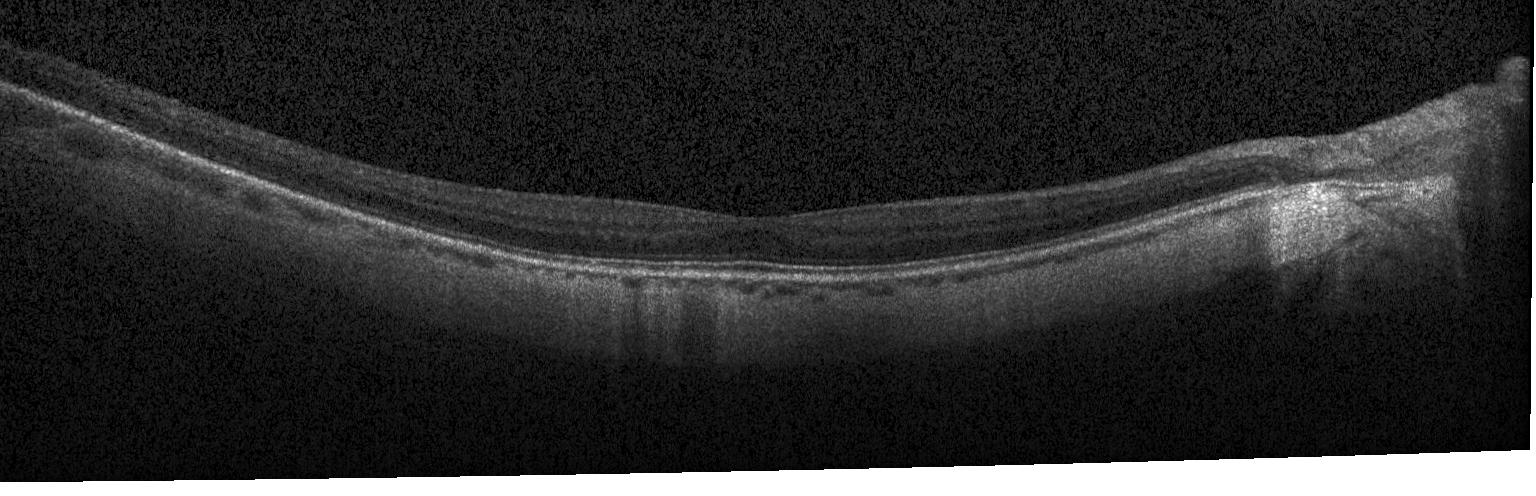
Finding: no CNV, DME, or drusen.